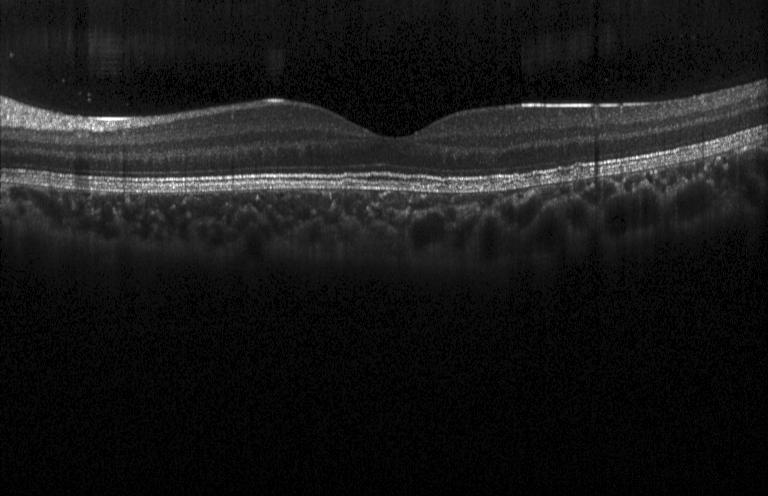
OCT line scan. Acquired on a Heidelberg Spectralis
No choroidal neovascularization, no diabetic macular edema, and no drusen.